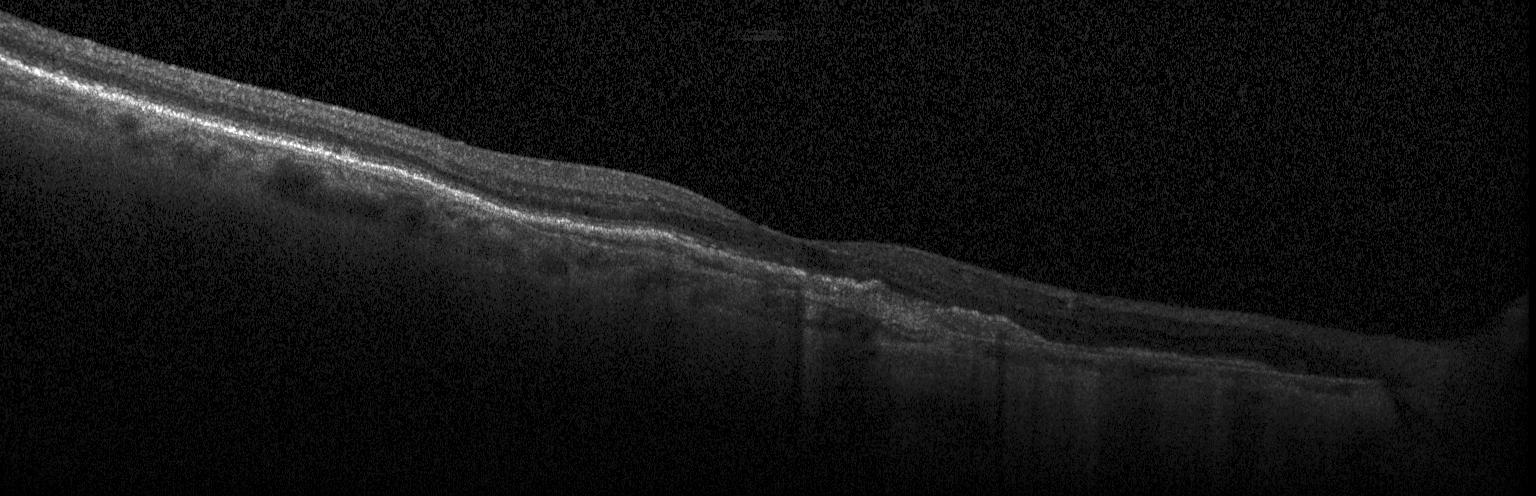
Through the macula · retinal OCT B-scan — A choroidal neovascular membrane.